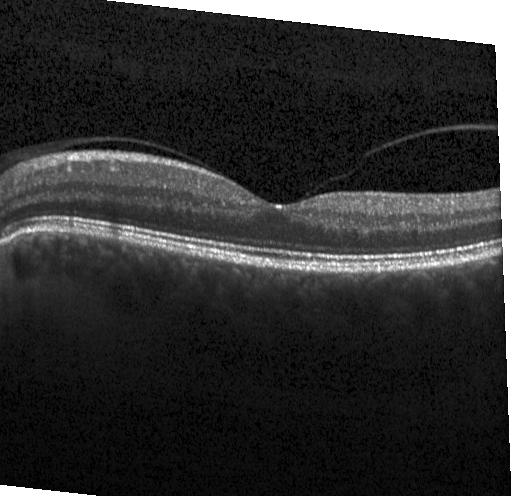 Retinal OCT B-scan, spectral-domain optical coherence tomography, centered on the fovea.
Macular OCT: no choroidal neovascularization, diabetic macular edema, or drusen.